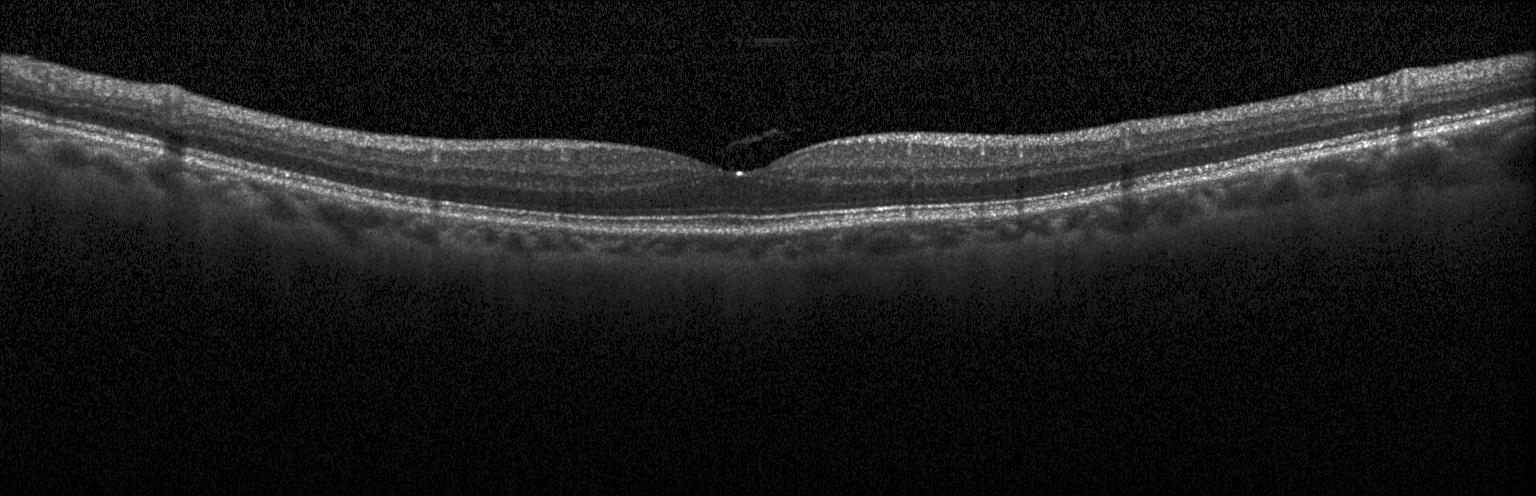 Retinal OCT B-scan — Diagnosis: no evidence of choroidal neovascularization, diabetic macular edema, or drusen.